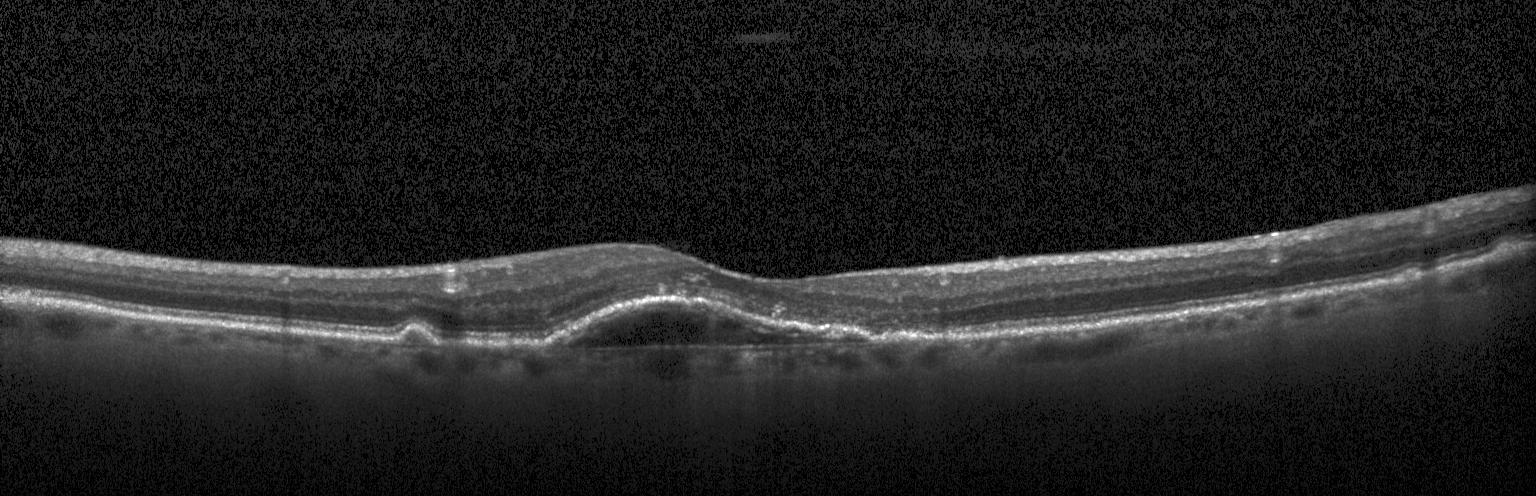 Retinal OCT B-scan.
Diagnosis: a choroidal neovascular membrane.